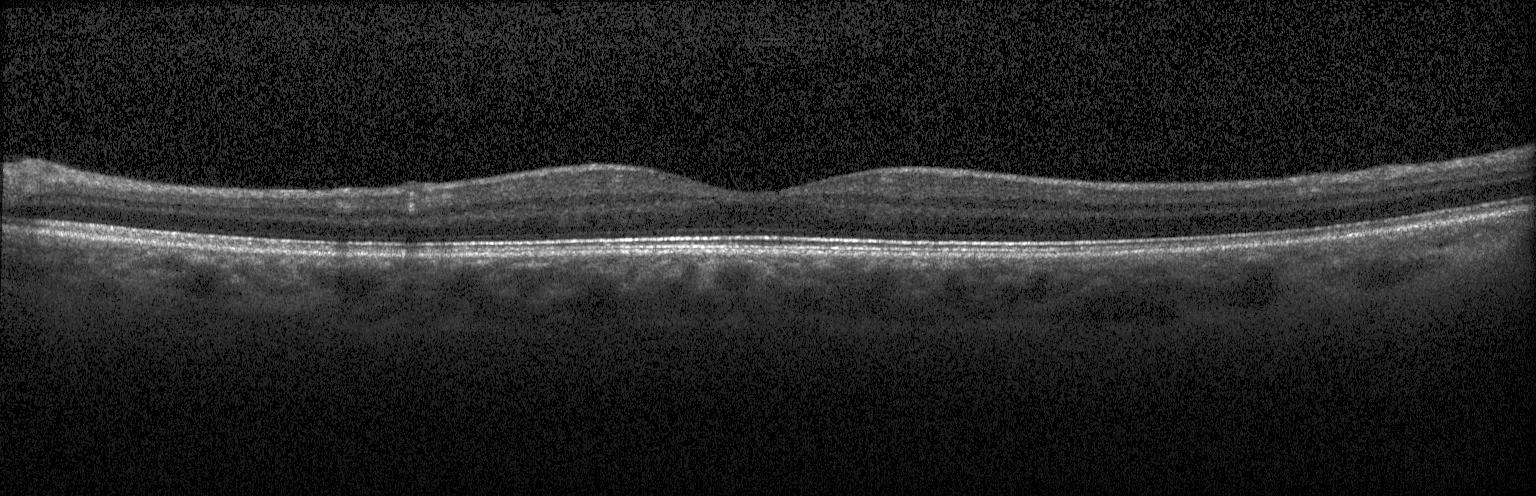
Macular OCT: no choroidal neovascularization, diabetic macular edema, or drusen.